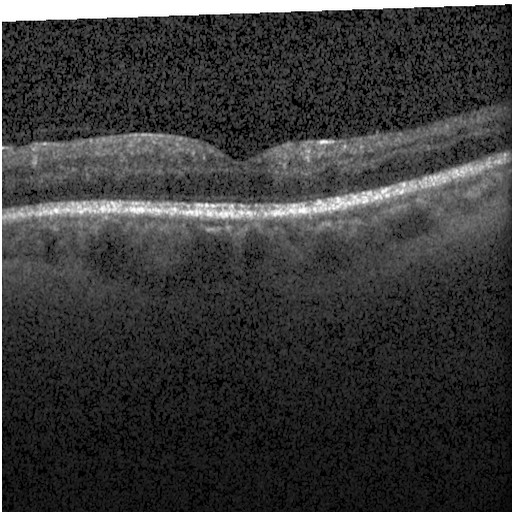

Macular OCT: diabetic macular edema.